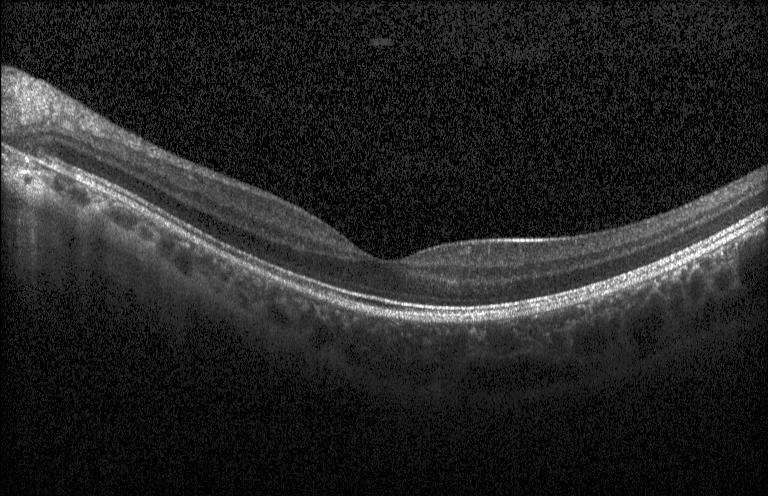

Instrument: Heidelberg Spectralis; through the macula; SD-OCT; retinal OCT B-scan — Assessment: no choroidal neovascularization, no diabetic macular edema, and no drusen.